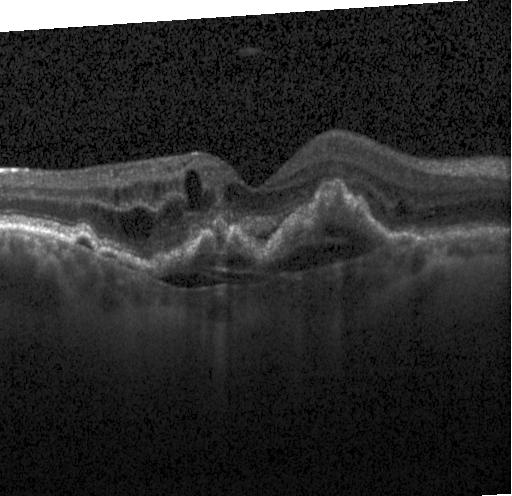
Spectral-domain optical coherence tomography; macular scan; OCT B-scan; Heidelberg Spectralis OCT system
The scan shows a choroidal neovascular membrane.